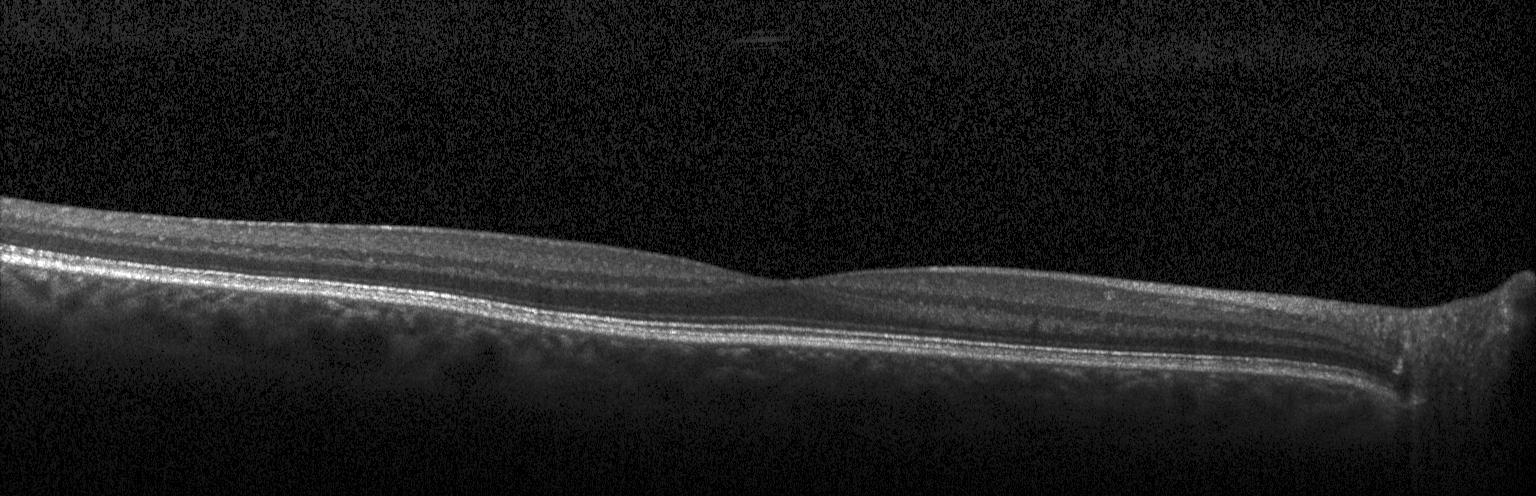

Optical coherence tomography B-scan, SD-OCT. OCT finding: no evidence of choroidal neovascularization, diabetic macular edema, or drusen.